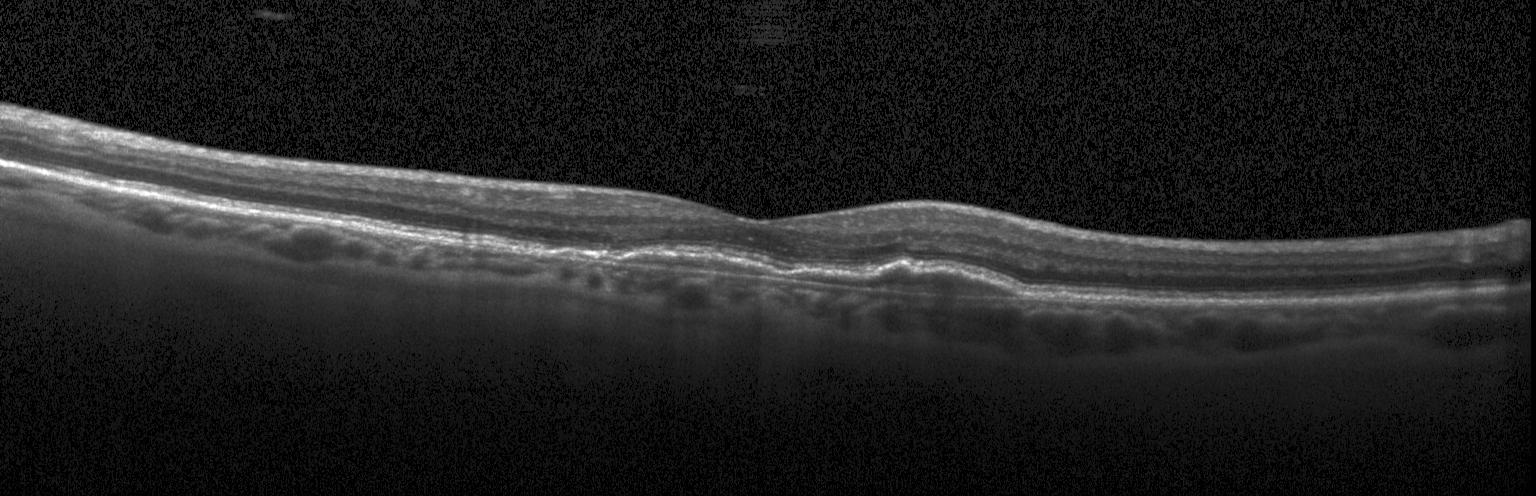

Diagnosis: a choroidal neovascular membrane.